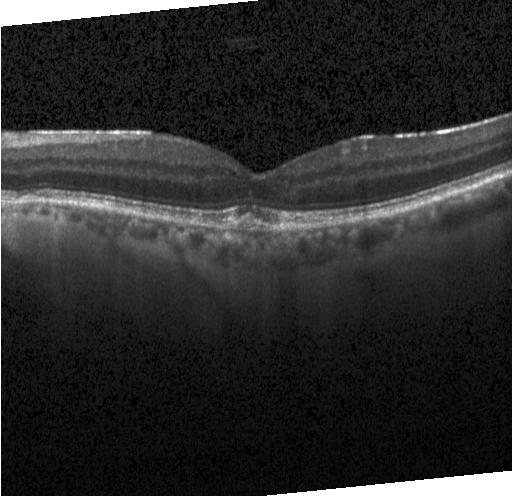 Macular OCT: a choroidal neovascular membrane.